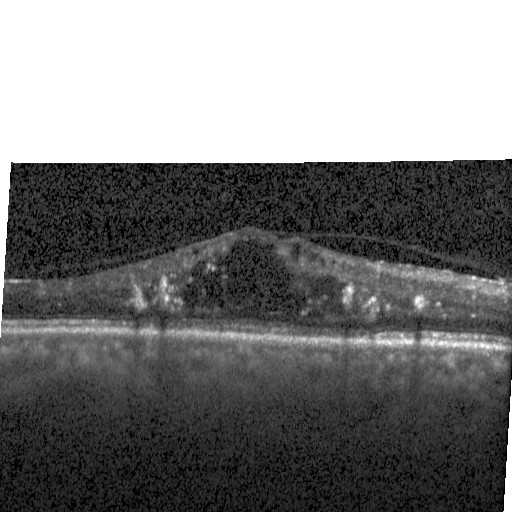 Through the macula. SD-OCT. Heidelberg Spectralis. Retinal OCT cross-section. Macular OCT: diabetic macular edema.